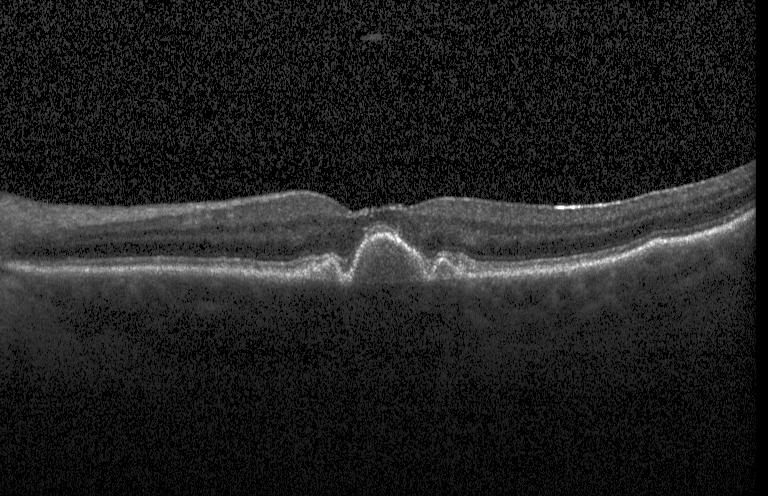 Heidelberg Spectralis. Retinal OCT B-scan
OCT finding: sub-RPE drusenoid deposits.